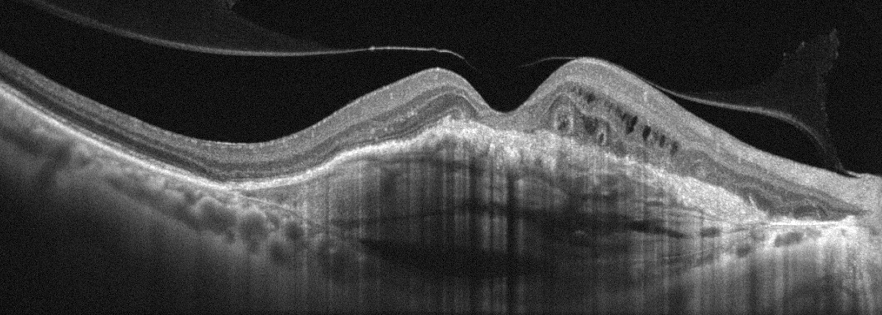
Macular OCT demonstrating AMD.